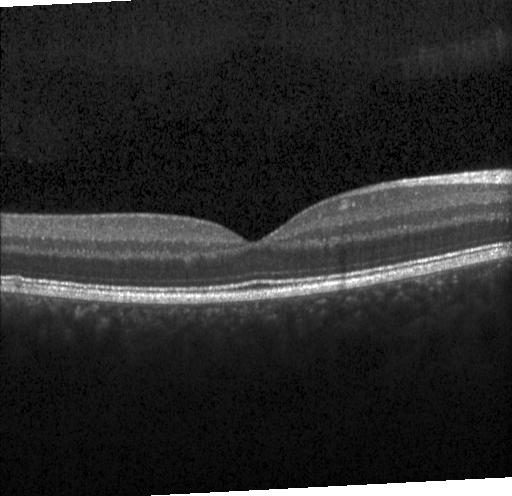
Spectral-domain optical coherence tomography, OCT B-scan — The scan shows neither choroidal neovascularization, diabetic macular edema, nor drusen.